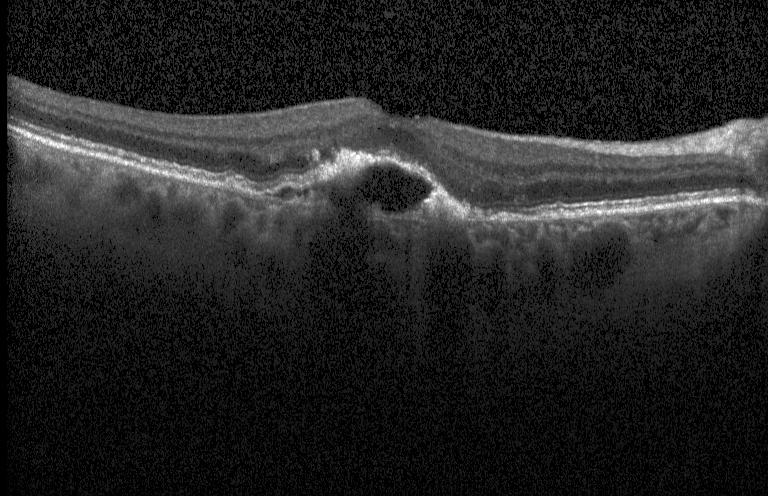
Centered on the fovea, retinal OCT cross-section — Dx: choroidal neovascularization (CNV).